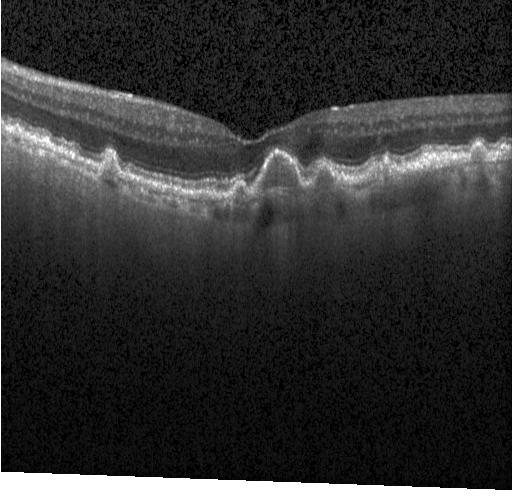
Macular OCT: drusen.